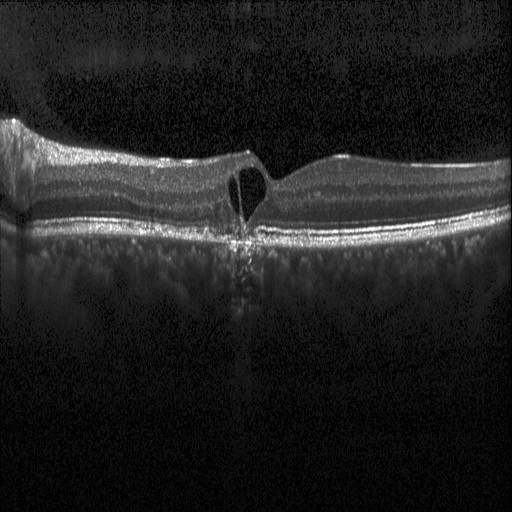 Spectral-domain OCT B-scan: DME.